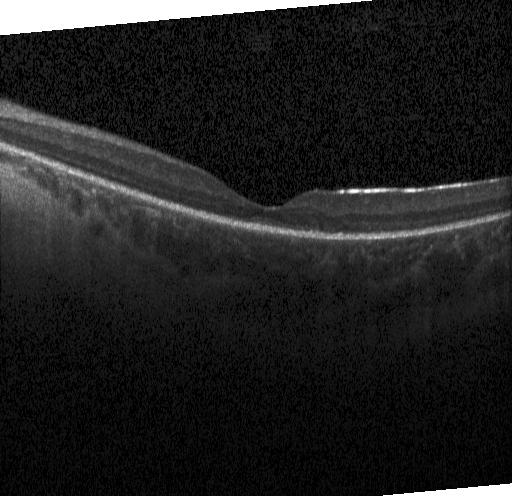
Diagnosis: no evidence of CNV, DME, or drusen.